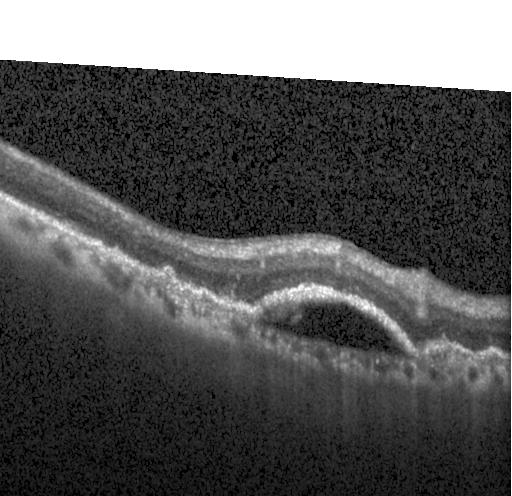

Finding: a choroidal neovascular membrane.